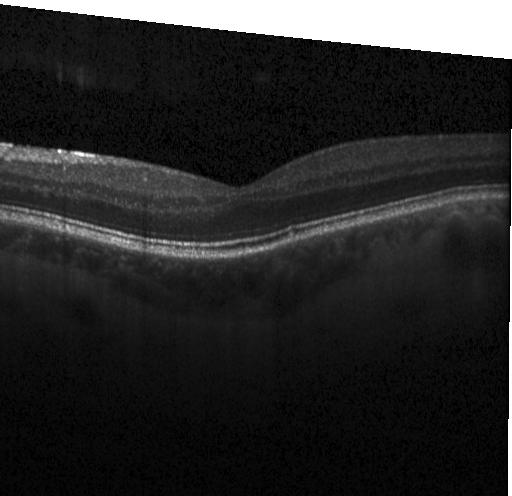
Optical coherence tomography scan · SD-OCT · Heidelberg Spectralis OCT system
The scan shows neither choroidal neovascularization, diabetic macular edema, nor drusen.